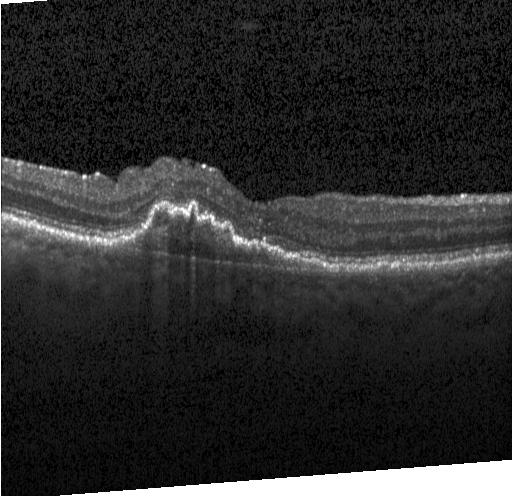 Instrument: Heidelberg Spectralis · retinal OCT B-scan · through the macula.
Impression: a choroidal neovascular membrane.